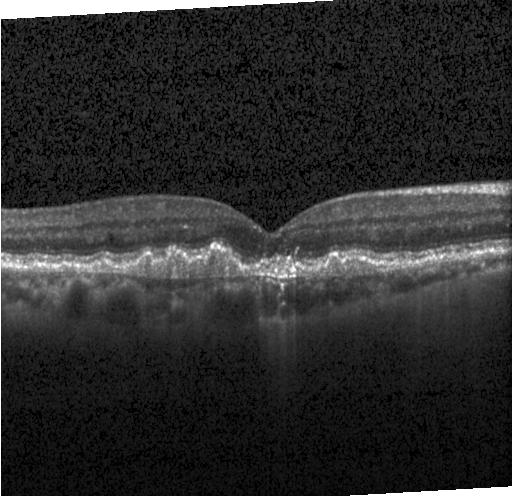
Dx: CNV.